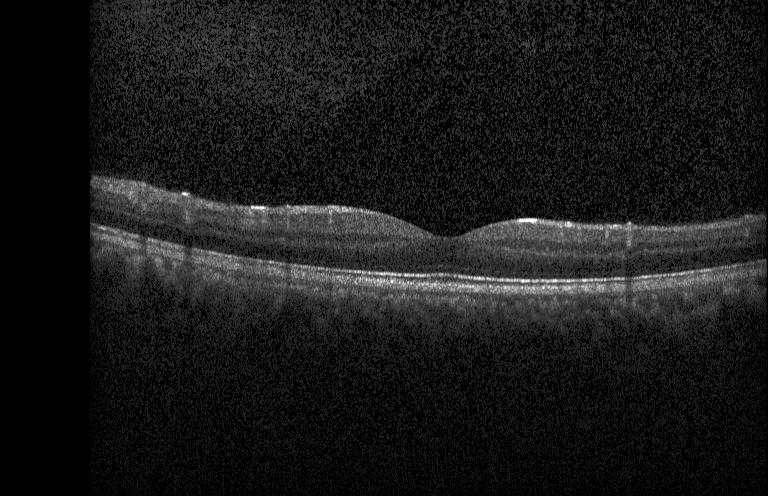 Spectral-domain optical coherence tomography · acquired on a Heidelberg Spectralis · horizontal scan through the fovea · OCT line scan
No CNV, no DME, and no drusen.